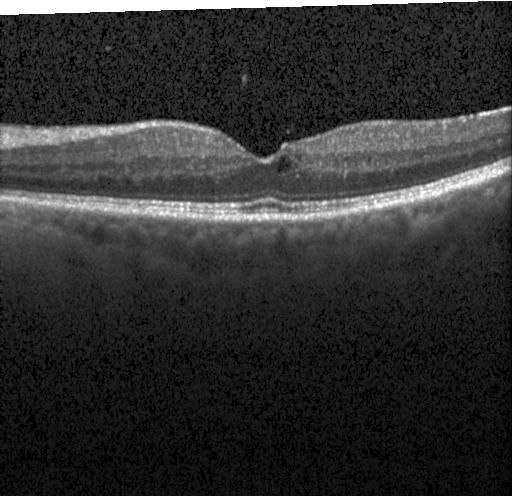

Horizontal scan through the fovea · spectral-domain optical coherence tomography · OCT B-scan
Diagnosis: diabetic macular edema.